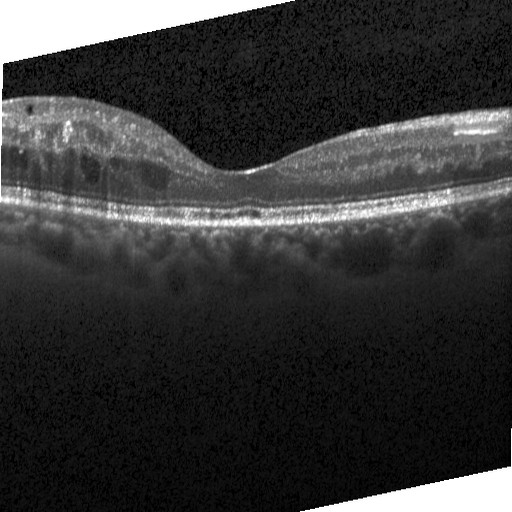
The scan shows DME.